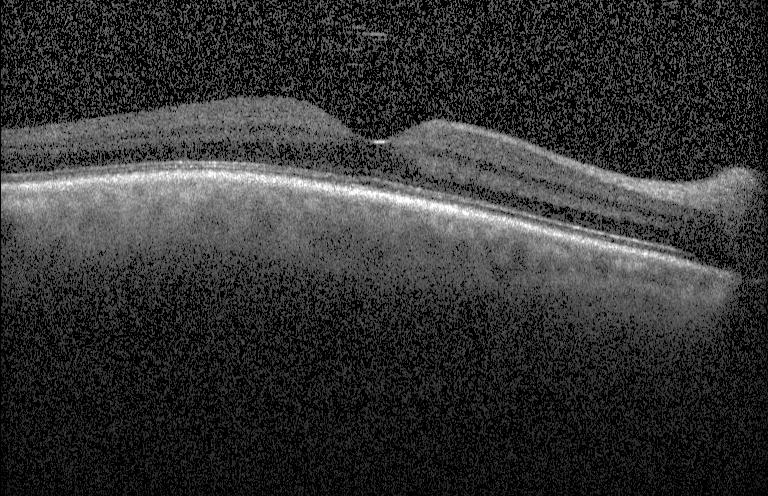

Through the macula; Heidelberg Spectralis; retinal OCT cross-section.
Impression: neither choroidal neovascularization, diabetic macular edema, nor drusen.